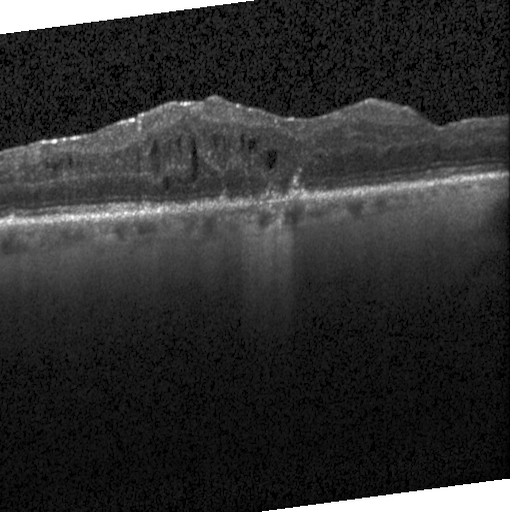 Centered on the fovea; spectral-domain OCT; retinal OCT cross-section. Diagnosis: diabetic macular edema (DME).